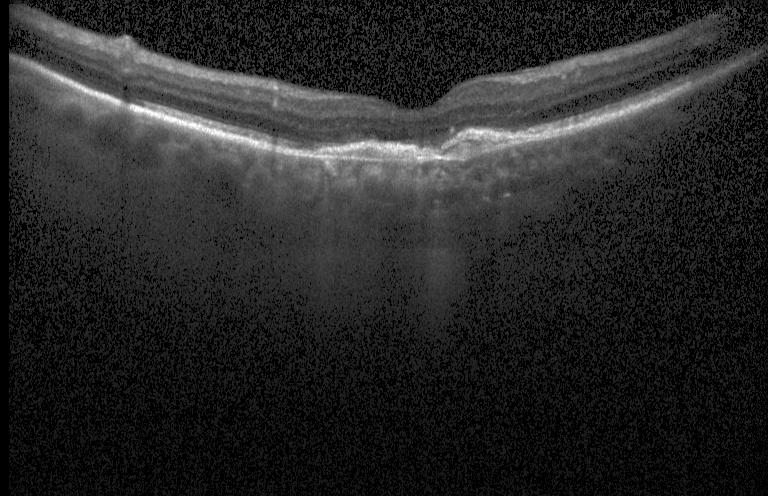 OCT scan showing choroidal neovascularization.